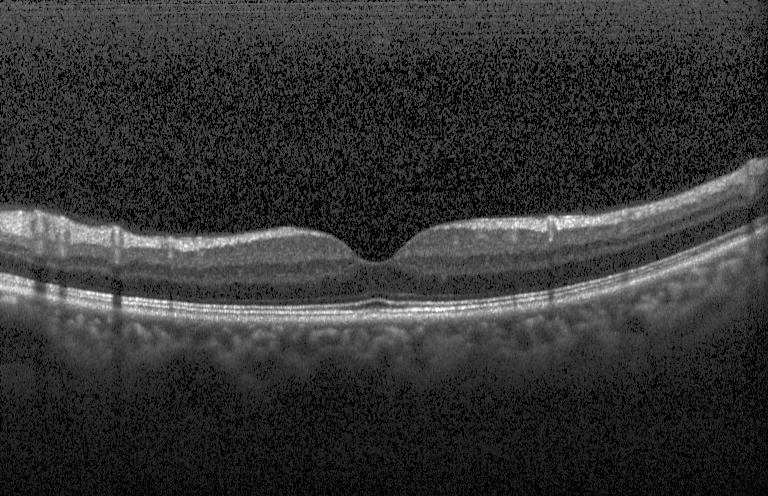 Macular OCT: no CNV, DME, or drusen.